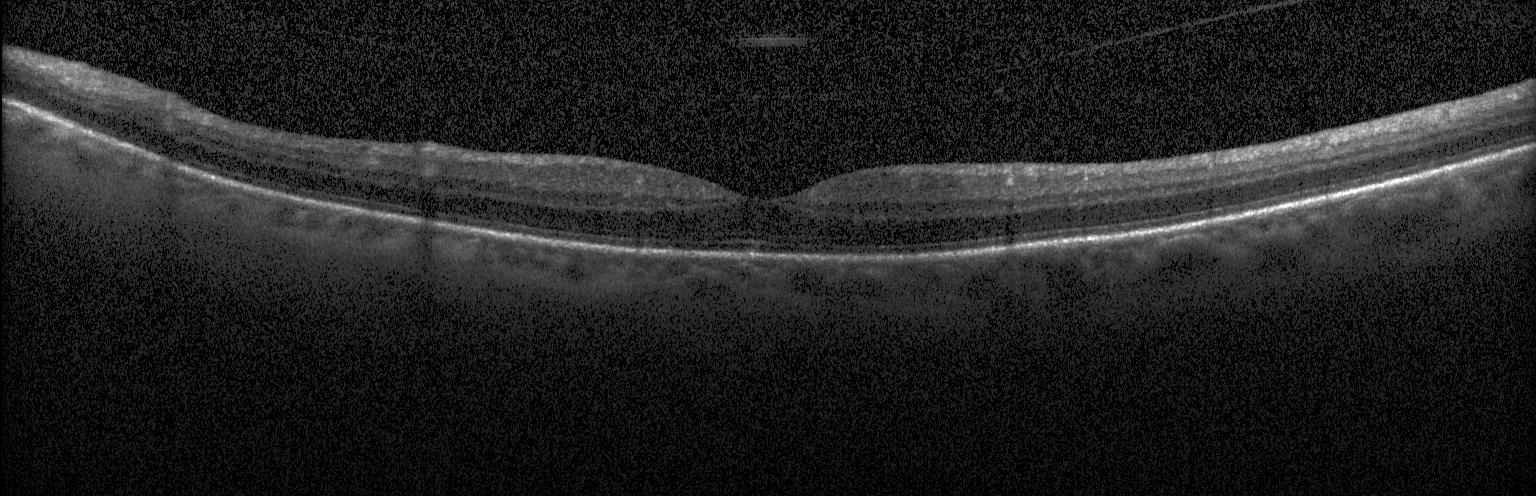 Centered on the fovea, optical coherence tomography B-scan, SD-OCT, acquired on a Heidelberg Spectralis
Finding: no choroidal neovascularization, no diabetic macular edema, and no drusen.